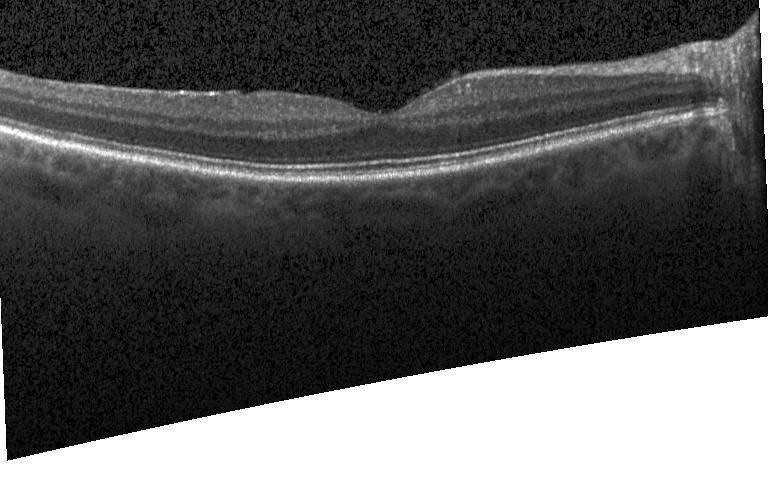 Heidelberg Spectralis. Retinal OCT cross-section. Centered on the fovea. Spectral-domain optical coherence tomography
Finding: neither choroidal neovascularization, diabetic macular edema, nor drusen.